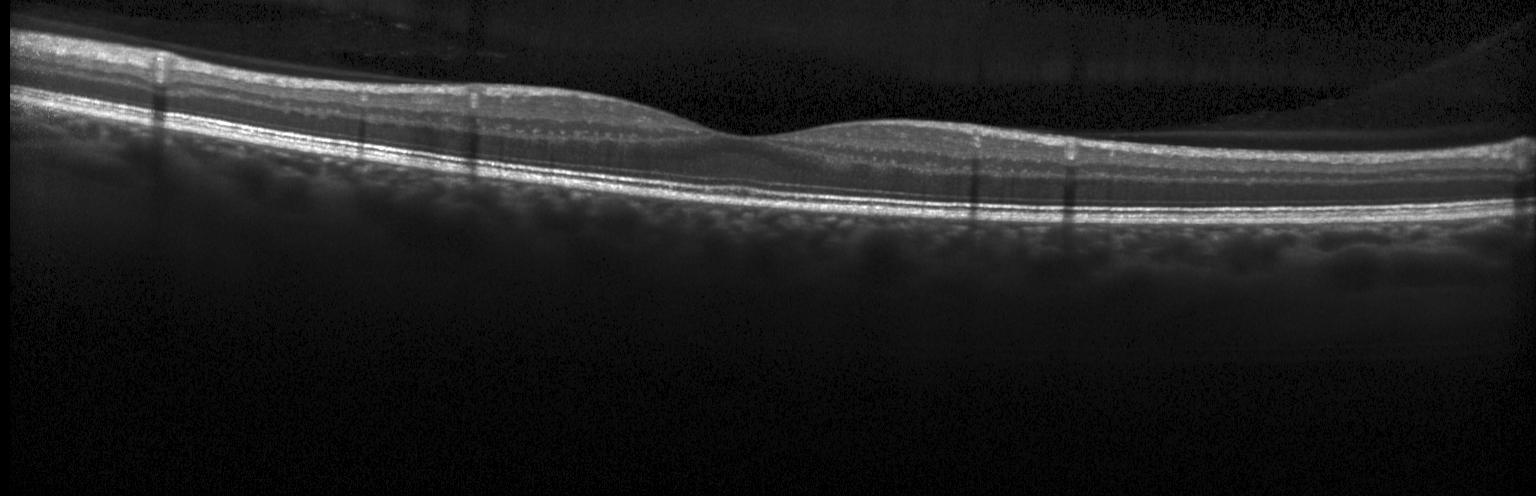 Heidelberg Spectralis OCT system. Macular scan. Spectral-domain OCT. Retinal OCT B-scan. Diagnosis: no choroidal neovascularization, diabetic macular edema, or drusen.